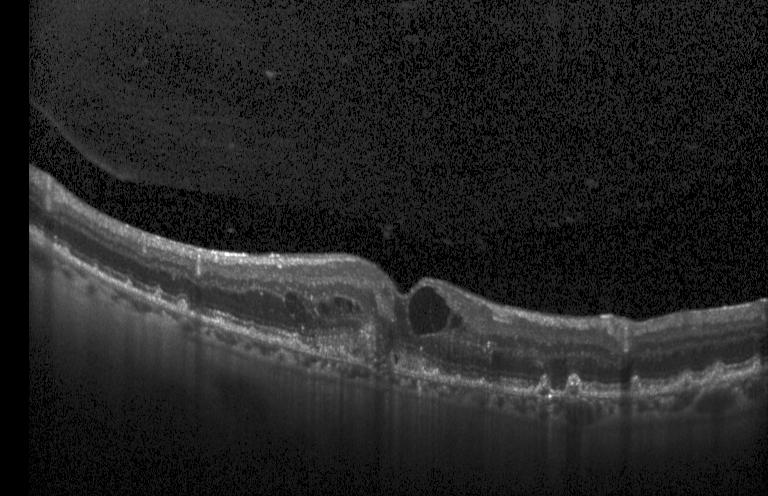 Optical coherence tomography B-scan. Through the macula. SD-OCT. Heidelberg Spectralis.
This B-scan demonstrates choroidal neovascularization (CNV).